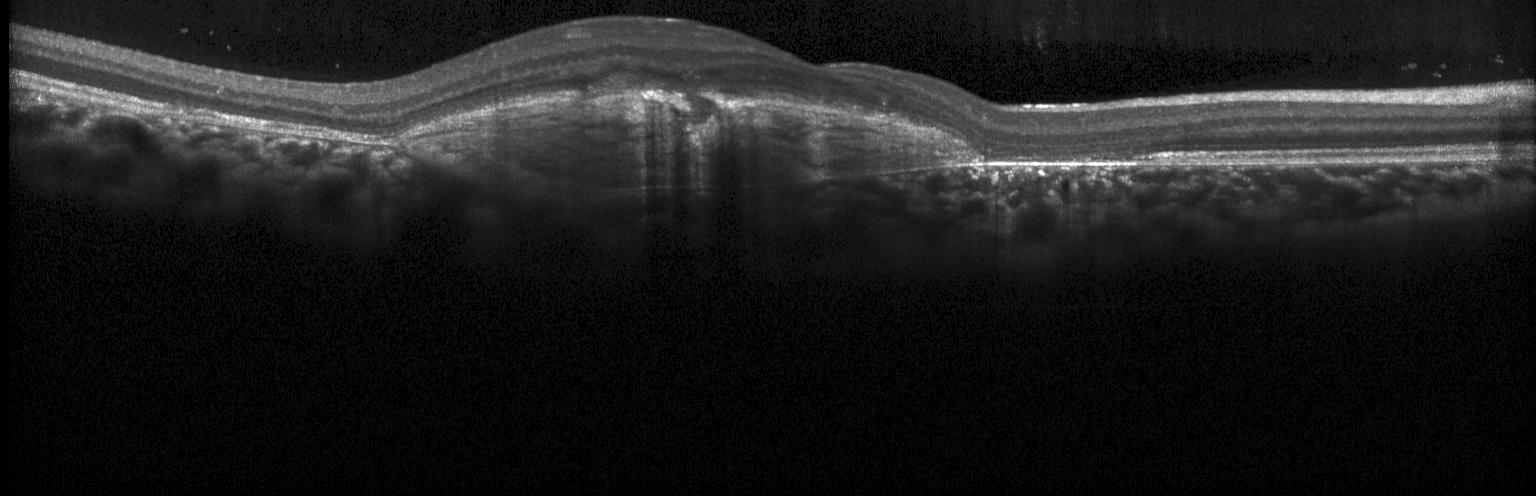

Fovea-centered · Heidelberg Spectralis · OCT line scan — Impression: a choroidal neovascular membrane.